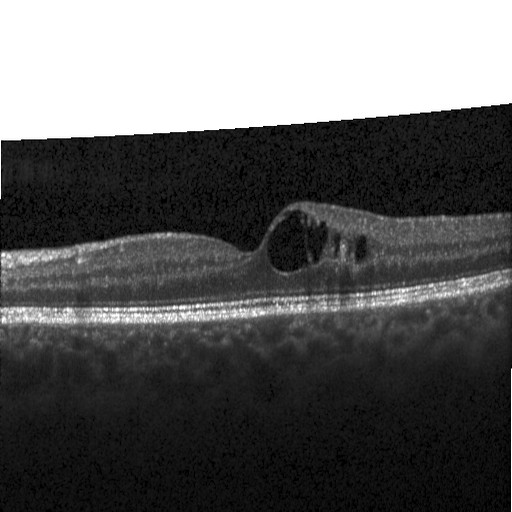
This B-scan demonstrates diabetic macular edema (DME).